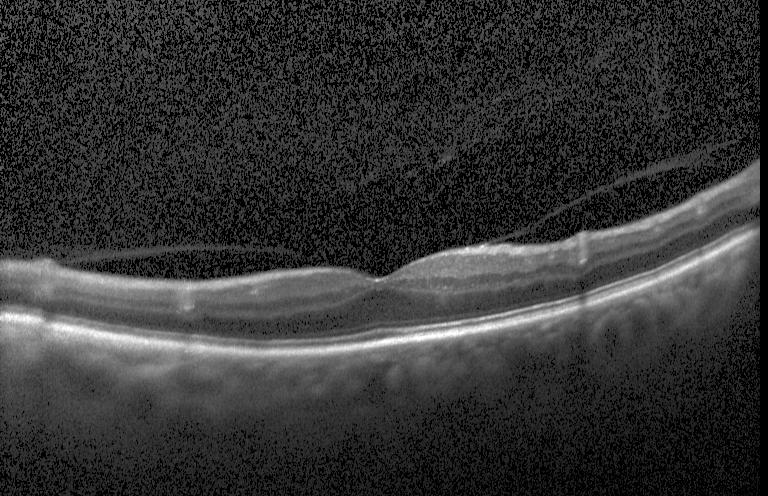 No choroidal neovascularization, diabetic macular edema, or drusen.